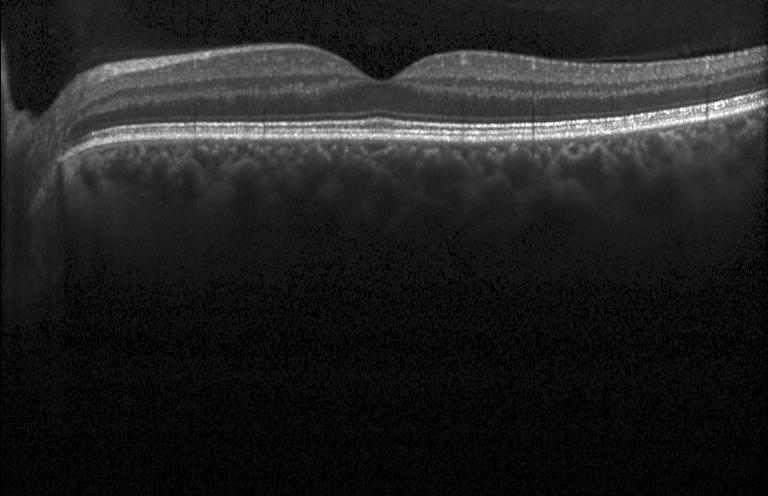
Impression: no CNV, no DME, and no drusen.